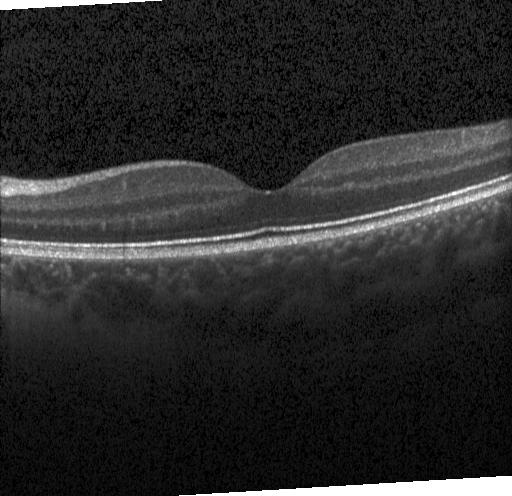

Retinal OCT cross-section; Heidelberg Spectralis OCT system; horizontal scan through the fovea — Finding: neither choroidal neovascularization, diabetic macular edema, nor drusen.